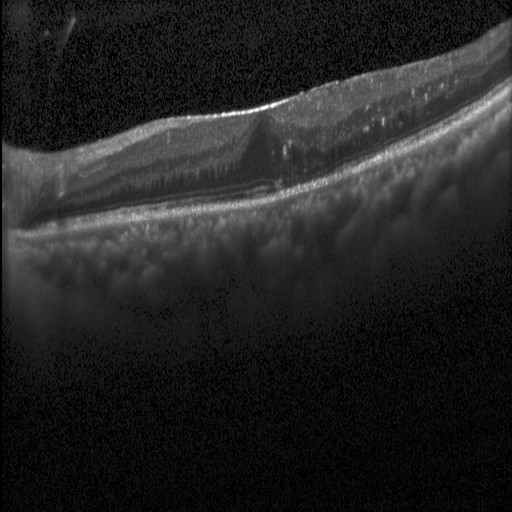
Retinal OCT B-scan; centered on the fovea; Heidelberg Spectralis; spectral-domain optical coherence tomography. Dx: diabetic macular edema (DME).